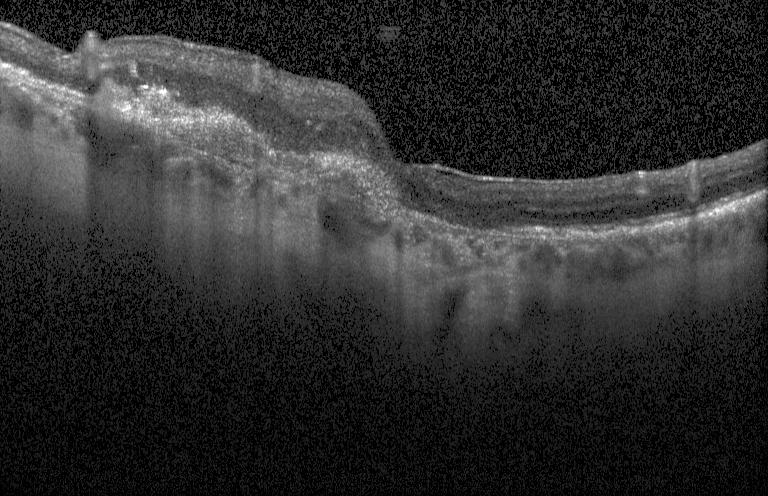

Retinal OCT B-scan; instrument: Heidelberg Spectralis; SD-OCT. The scan shows CNV.